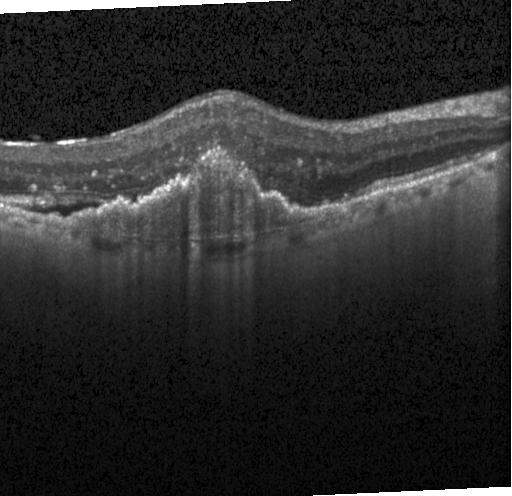 Macular scan; OCT line scan.
Dx: CNV.